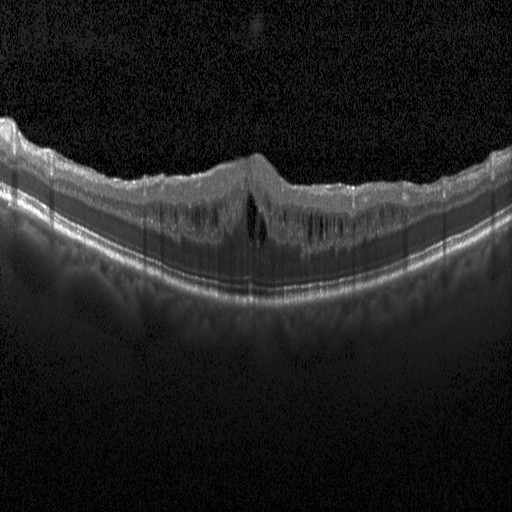
The scan shows DME.